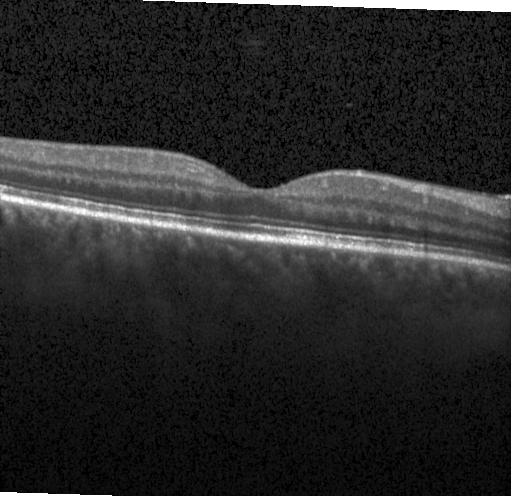 Spectral-domain OCT · optical coherence tomography B-scan · acquired on a Heidelberg Spectralis — Dx: no evidence of CNV, DME, or drusen.